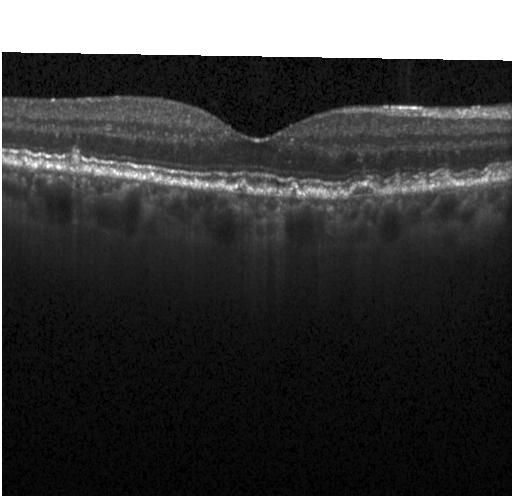
OCT finding: multiple drusen.